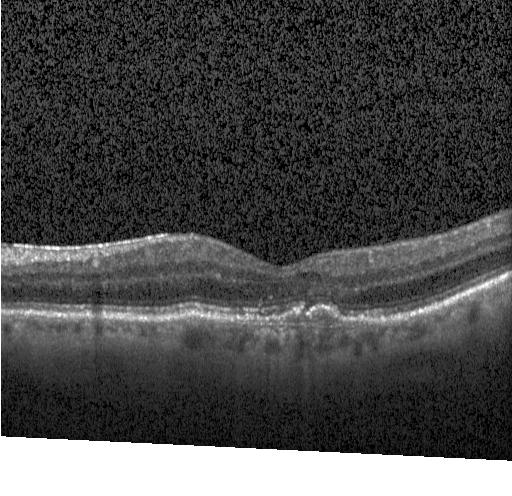 OCT B-scan
Diagnosis: CNV.